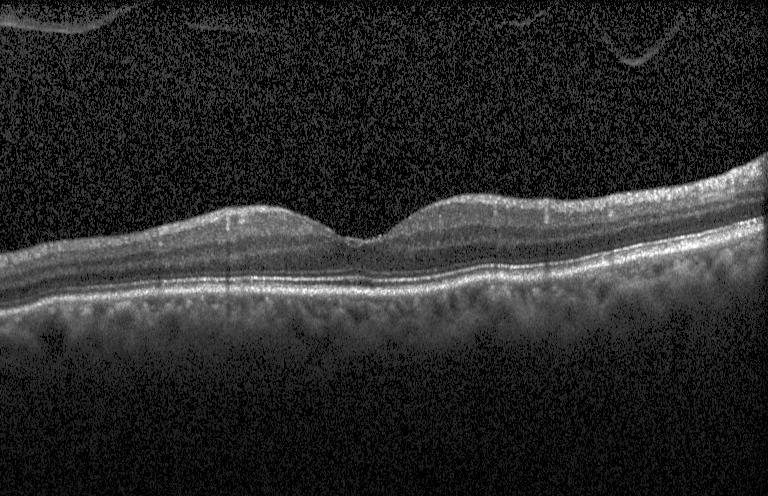
Macular scan · acquired on a Heidelberg Spectralis · spectral-domain OCT · OCT B-scan.
Diagnosis: no choroidal neovascularization, diabetic macular edema, or drusen.